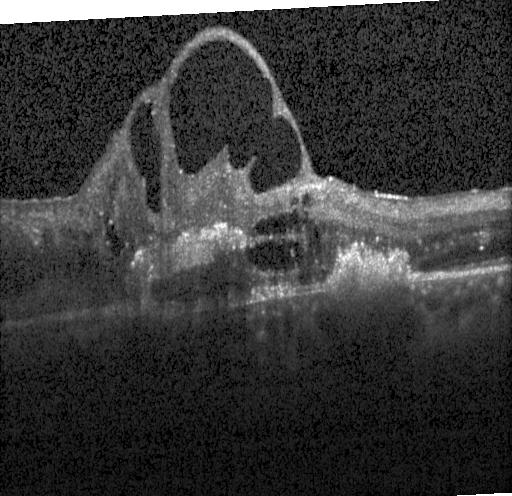 Finding: choroidal neovascularization.